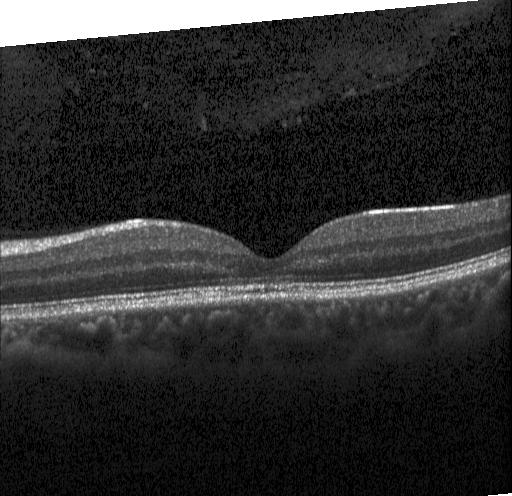

Retinal OCT cross-section showing no choroidal neovascularization, diabetic macular edema, or drusen.